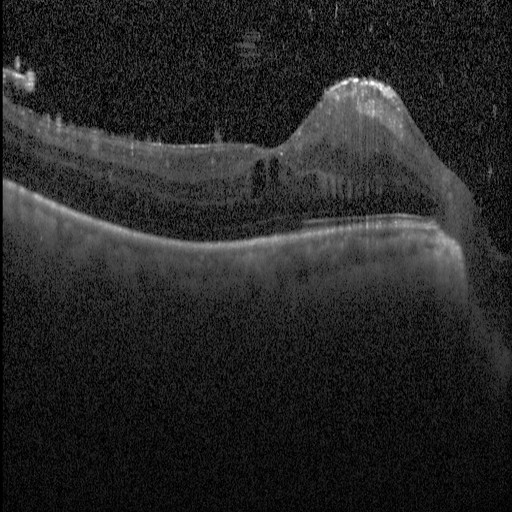

OCT B-scan showing diabetic macular edema (DME).